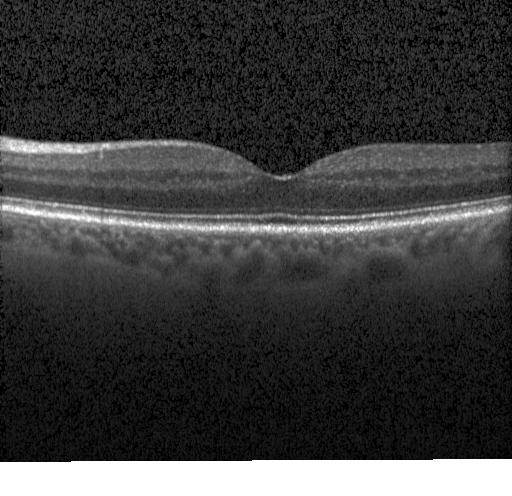 The scan shows no choroidal neovascularization, no diabetic macular edema, and no drusen.